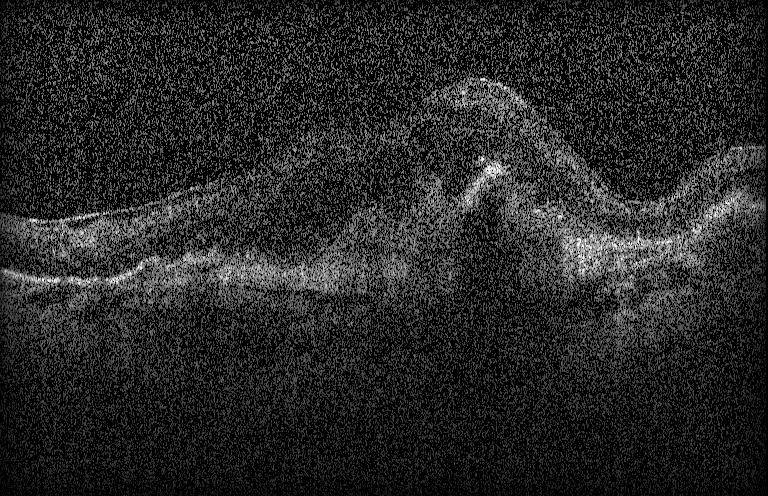
OCT finding: choroidal neovascularization.